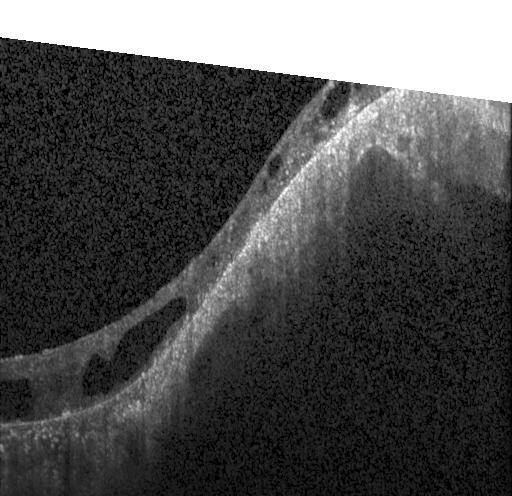 Impression: DME.